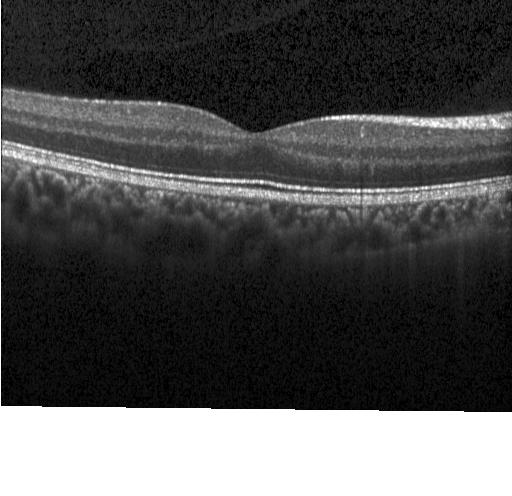 OCT finding: no CNV, DME, or drusen.